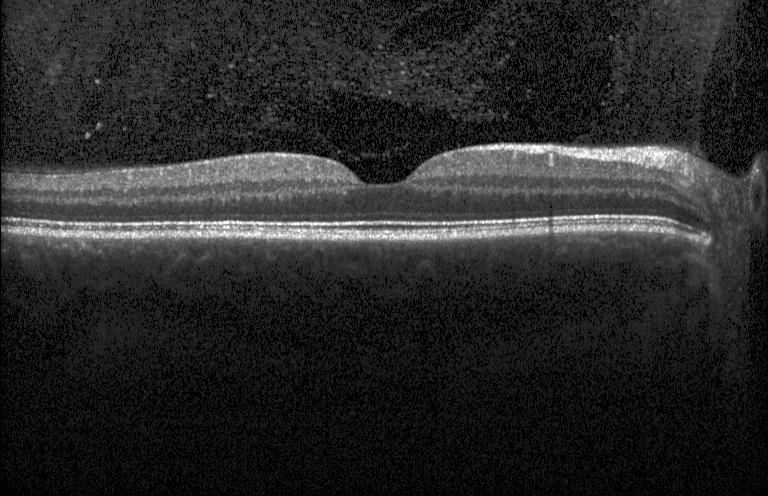
Optical coherence tomography scan.
Diagnosis: no choroidal neovascularization, no diabetic macular edema, and no drusen.